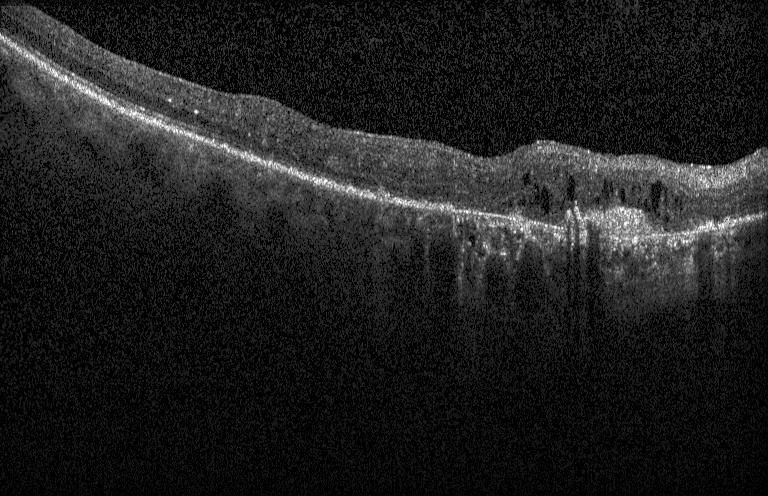
Retinal OCT B-scan, spectral-domain optical coherence tomography
Finding: a choroidal neovascular membrane.